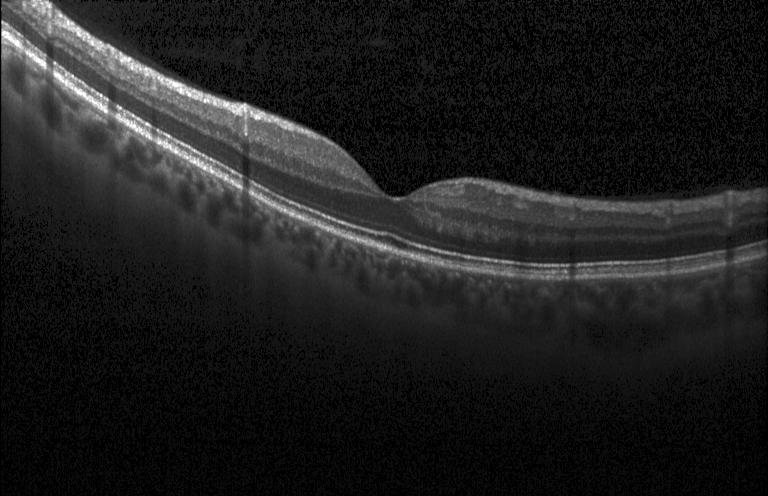 Macular OCT demonstrating no CNV, DME, or drusen.